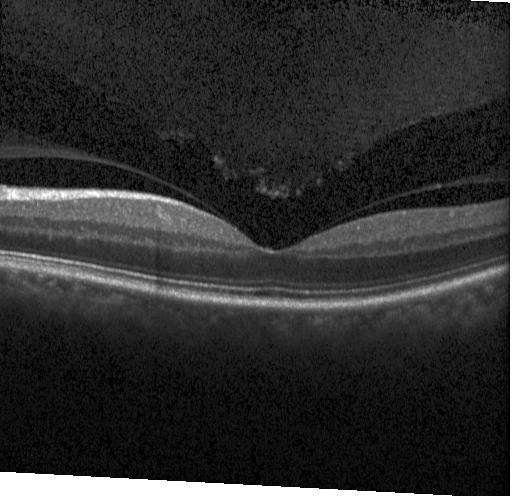

Diagnosis: no evidence of CNV, DME, or drusen.